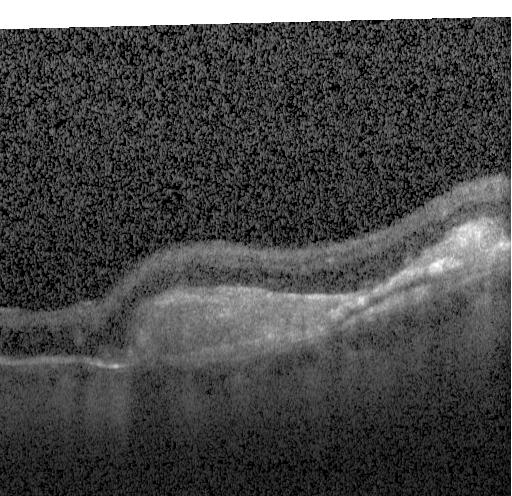 Spectral-domain OCT. Fovea-centered. Optical coherence tomography scan. Choroidal neovascularization (CNV).